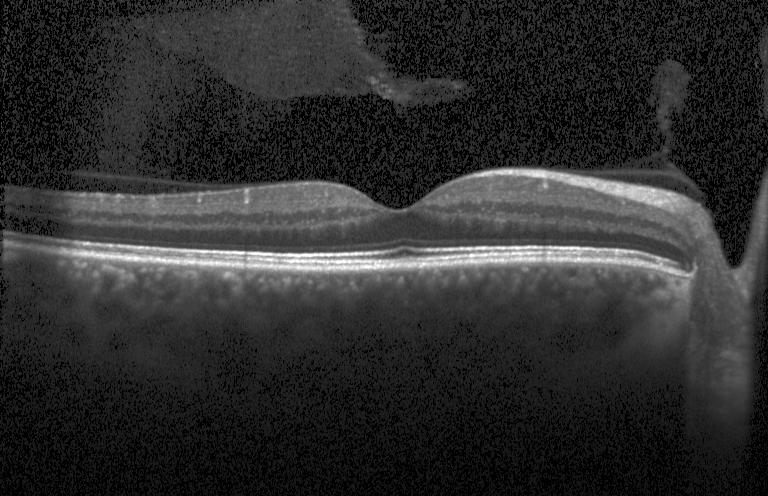 Macular scan · Heidelberg Spectralis OCT system · retinal OCT B-scan. Finding: neither choroidal neovascularization, diabetic macular edema, nor drusen.